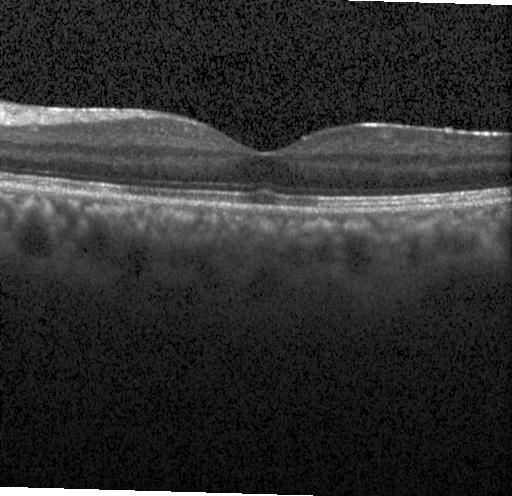
Through the macula, retinal OCT cross-section. Diagnosis: neither CNV, DME, nor drusen.